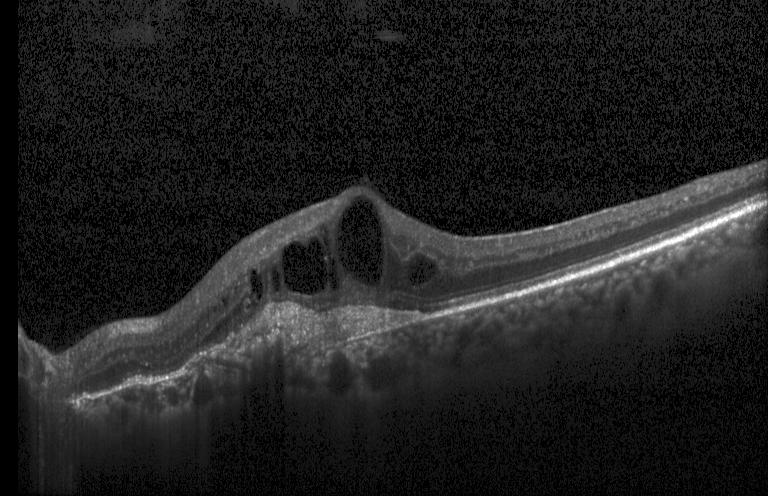

OCT line scan.
Finding: choroidal neovascularization (CNV).